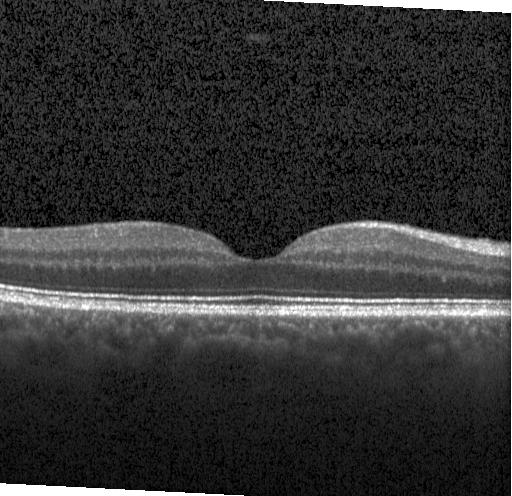

Impression: no evidence of CNV, DME, or drusen.